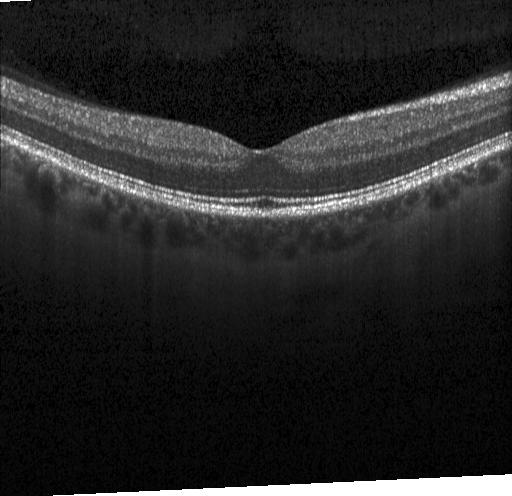

Assessment: no evidence of CNV, DME, or drusen.